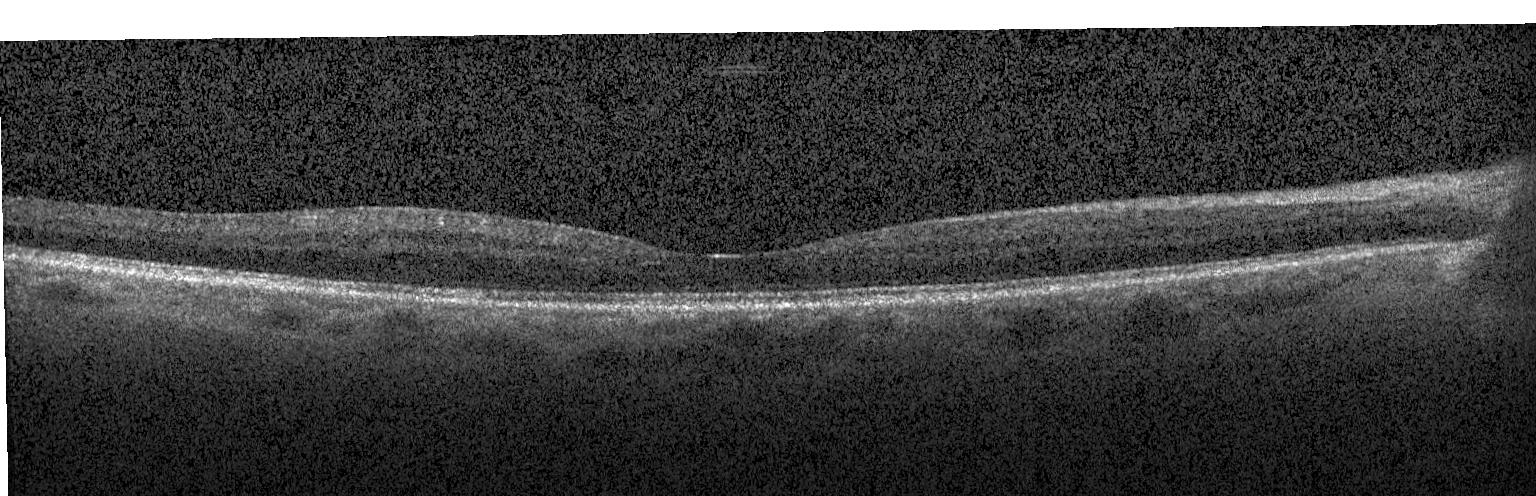 SD-OCT · retinal OCT cross-section — OCT finding: no evidence of choroidal neovascularization, diabetic macular edema, or drusen.